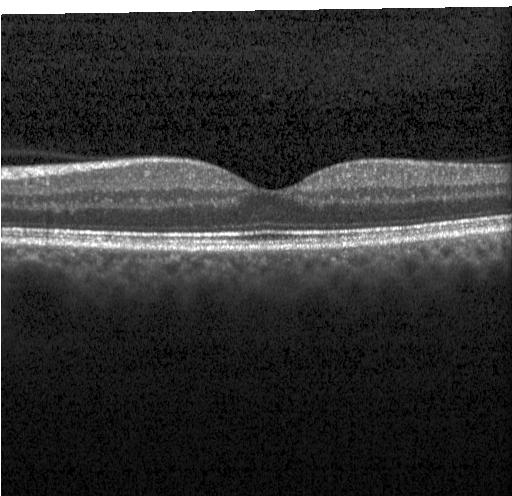 Heidelberg Spectralis. Retinal OCT B-scan.
Finding: no choroidal neovascularization, no diabetic macular edema, and no drusen.